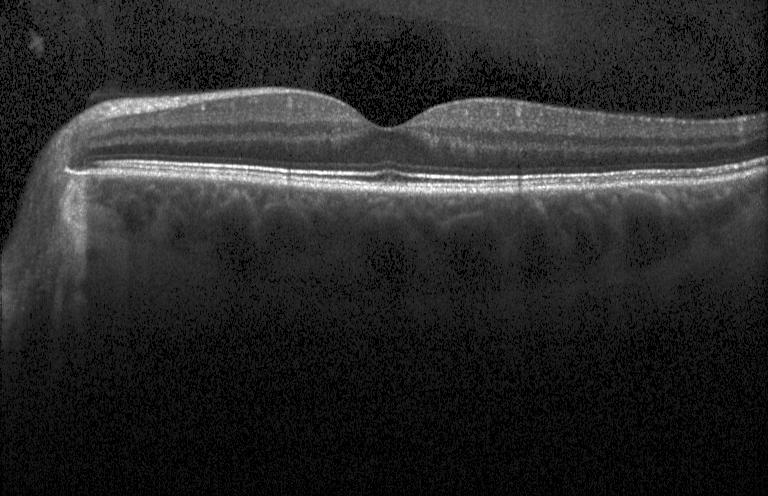 Retinal OCT B-scan. Macular scan. Acquired on a Heidelberg Spectralis — OCT finding: no evidence of choroidal neovascularization, diabetic macular edema, or drusen.